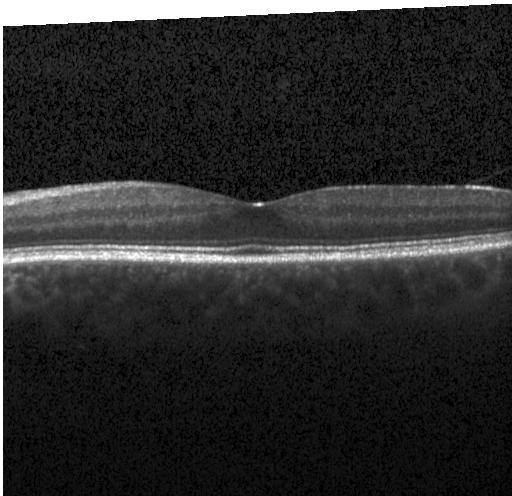
OCT scan showing no evidence of CNV, DME, or drusen.